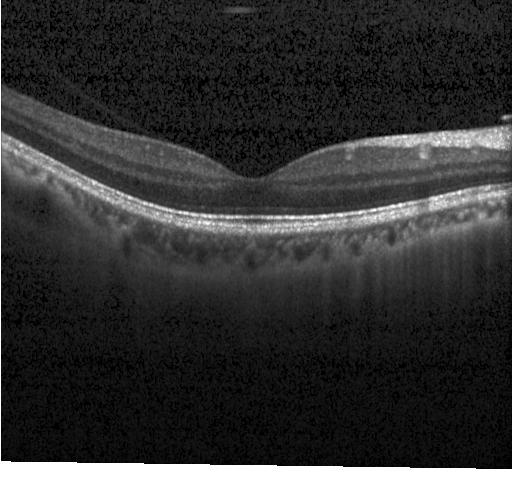 Heidelberg Spectralis OCT system. Optical coherence tomography scan.
Diagnosis: no evidence of choroidal neovascularization, diabetic macular edema, or drusen.